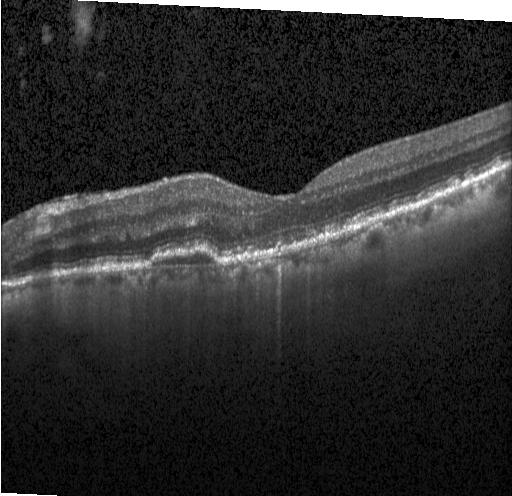
Spectral-domain optical coherence tomography; optical coherence tomography scan.
Dx: CNV.